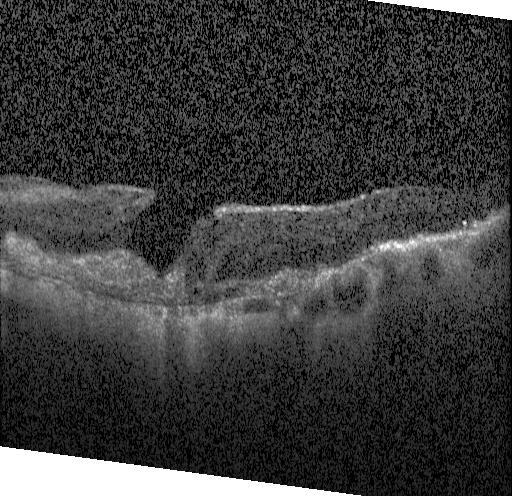 OCT line scan. Instrument: Heidelberg Spectralis. Assessment: a choroidal neovascular membrane.